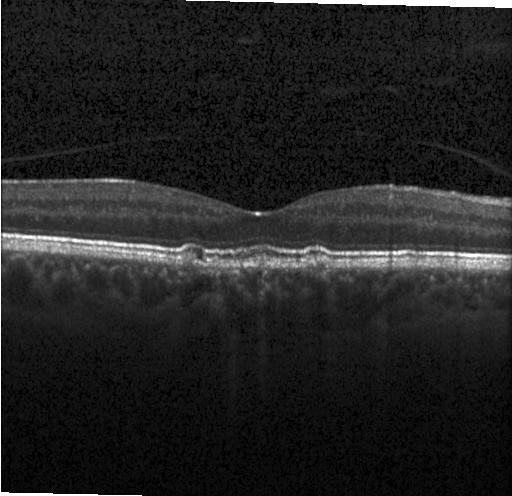 Macular OCT demonstrating sub-RPE drusenoid deposits.